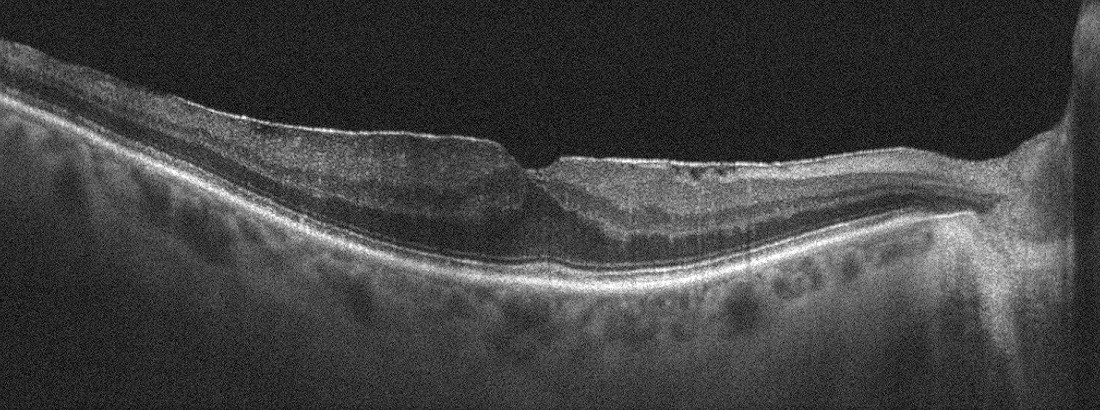 OCT B-scan. Optovue Avanti RTVue XR. Macular scan
Epiretinal membrane.